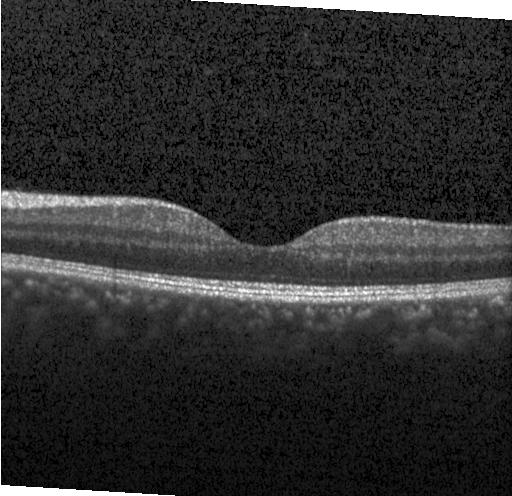
Finding: neither choroidal neovascularization, diabetic macular edema, nor drusen.